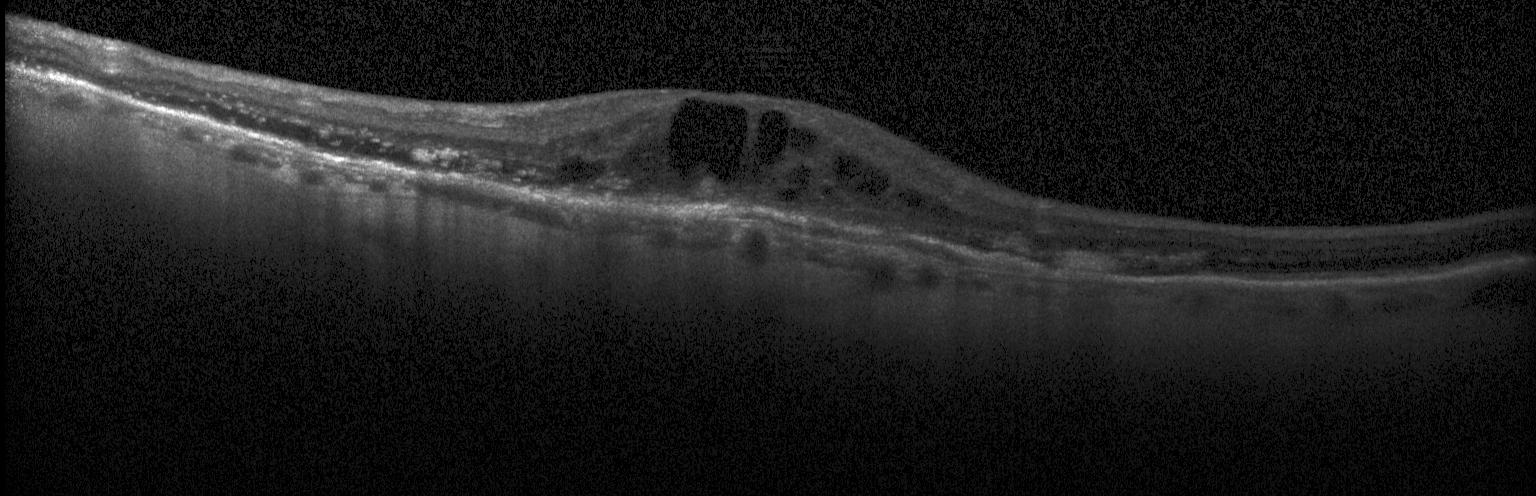 Fovea-centered · OCT line scan · Heidelberg Spectralis · spectral-domain optical coherence tomography — Diagnosis: a choroidal neovascular membrane.